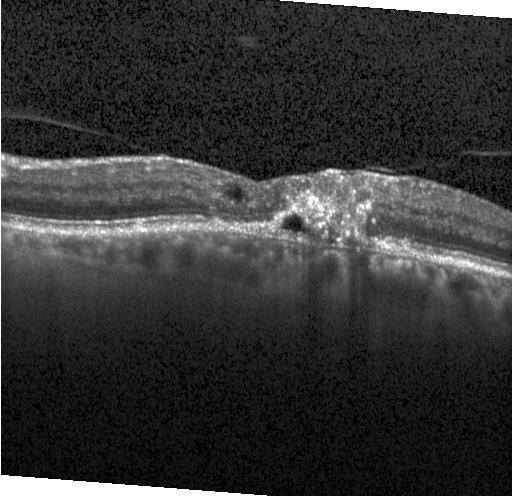

Impression: choroidal neovascularization (CNV).